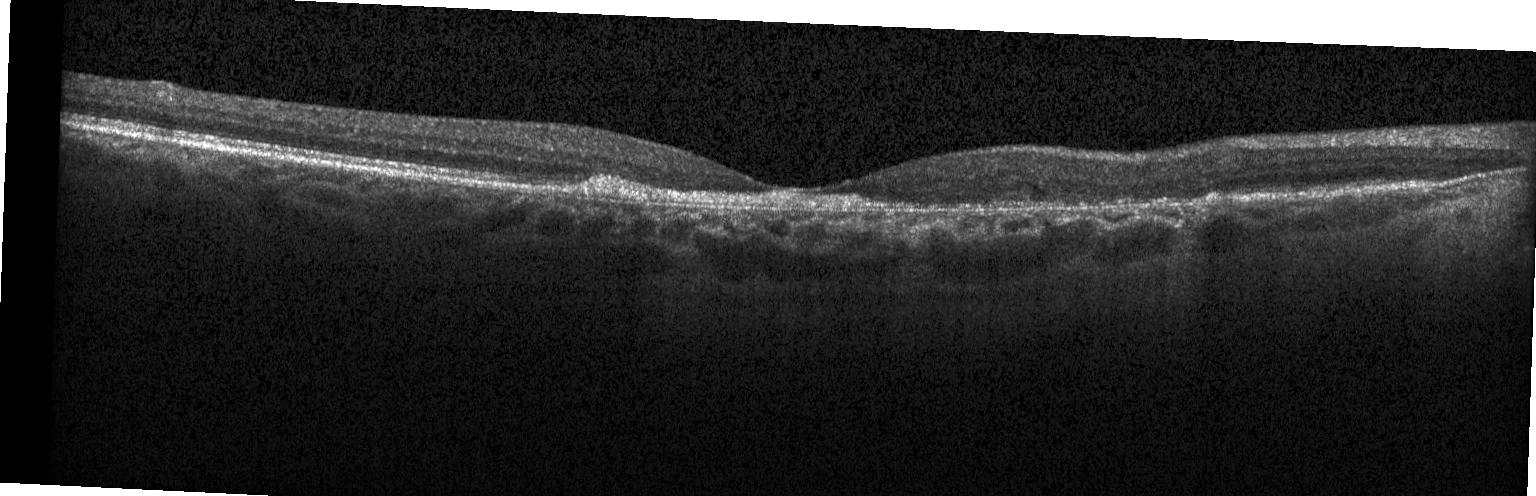
The scan shows choroidal neovascularization (CNV).